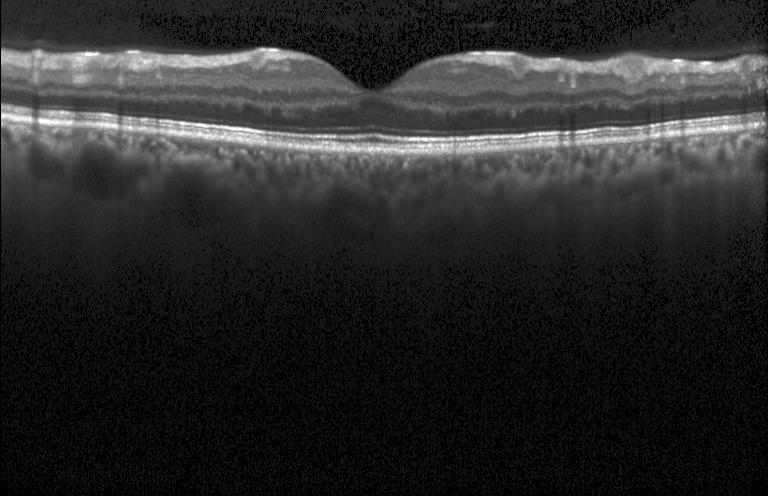

Finding: no evidence of CNV, DME, or drusen.